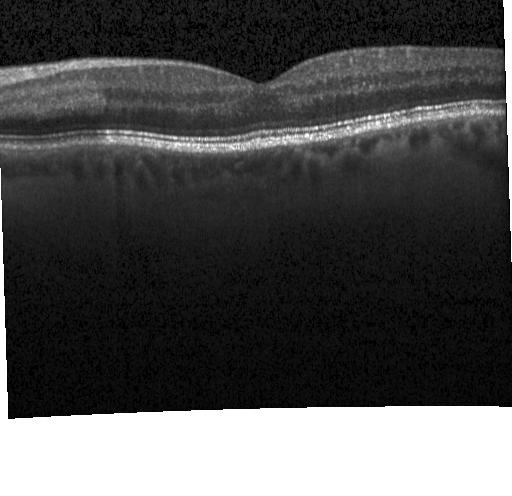

Fovea-centered · optical coherence tomography scan — Assessment: neither choroidal neovascularization, diabetic macular edema, nor drusen.